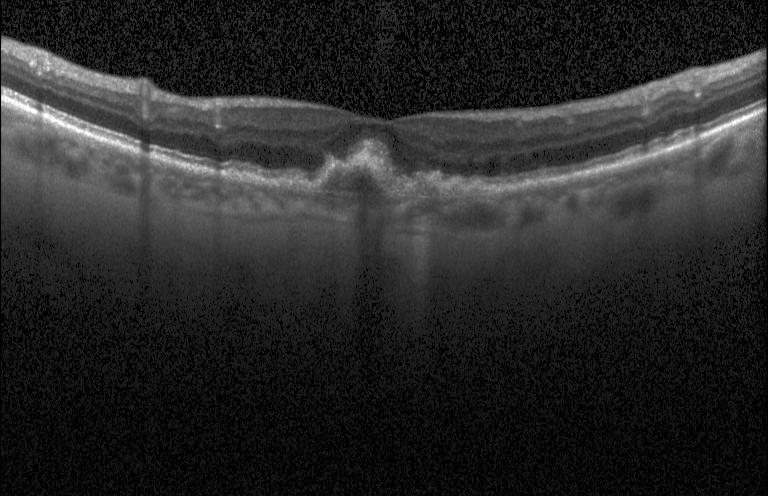
Impression: choroidal neovascularization (CNV).